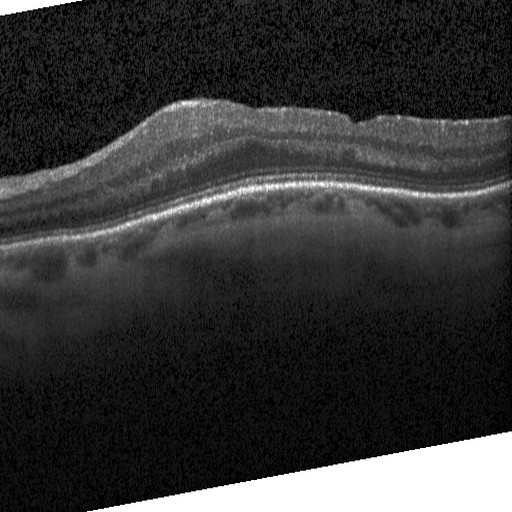
Finding: DME.